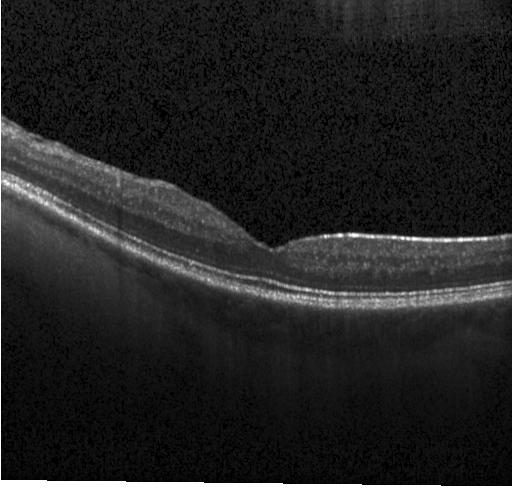 Retinal OCT B-scan.
Assessment: no CNV, no DME, and no drusen.